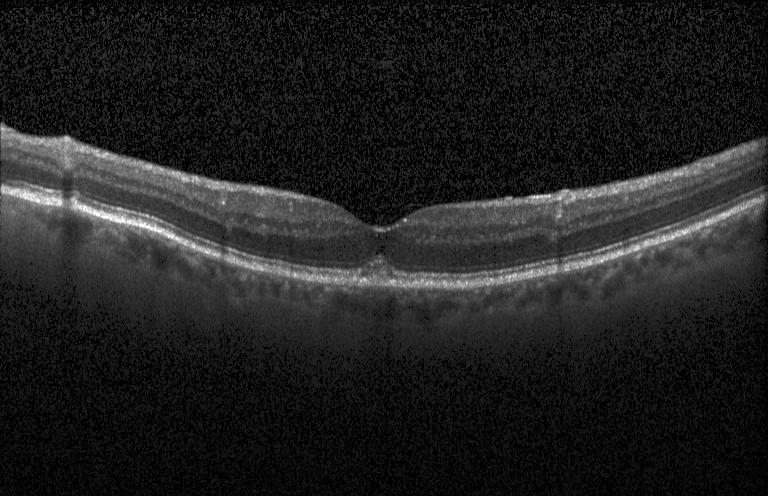

Retinal OCT cross-section · spectral-domain OCT · horizontal scan through the fovea. Sub-RPE drusenoid deposits.